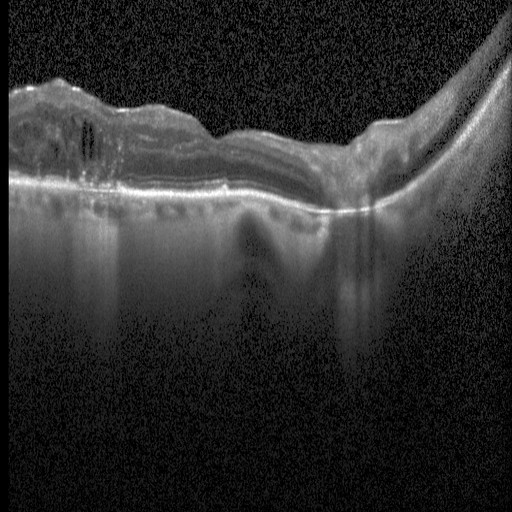 Spectral-domain OCT; optical coherence tomography B-scan; instrument: Heidelberg Spectralis.
Finding: DME.